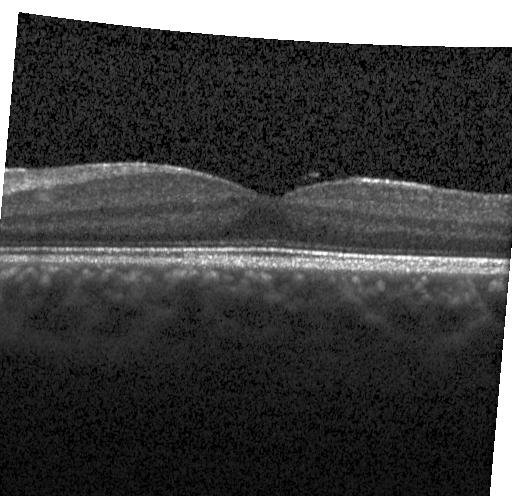
Finding: no choroidal neovascularization, diabetic macular edema, or drusen.